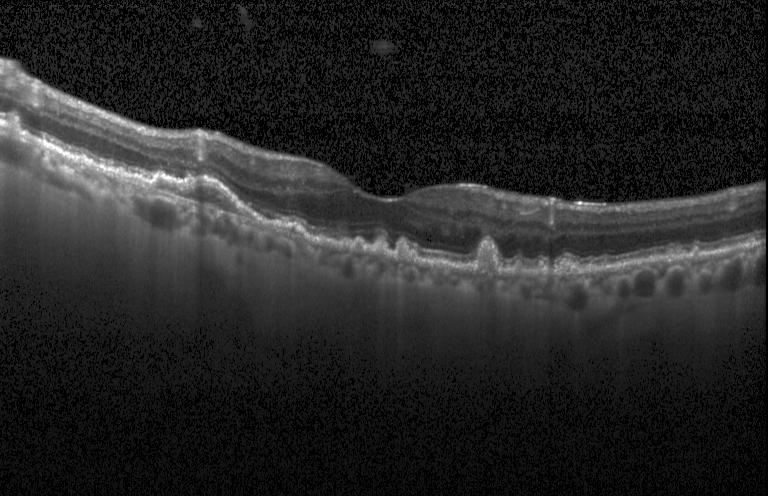
Dx: drusen.